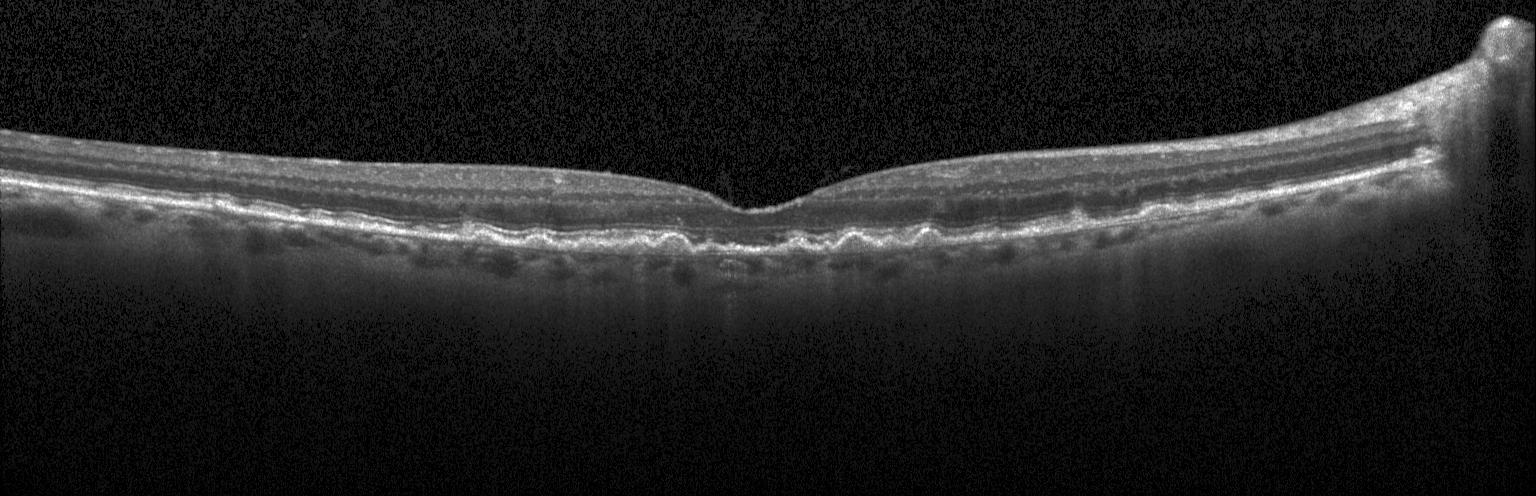

Retinal OCT cross-section showing sub-RPE drusenoid deposits.